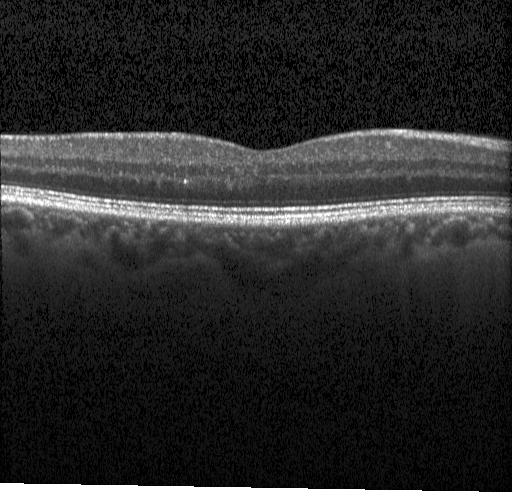 OCT B-scan showing no choroidal neovascularization, no diabetic macular edema, and no drusen.